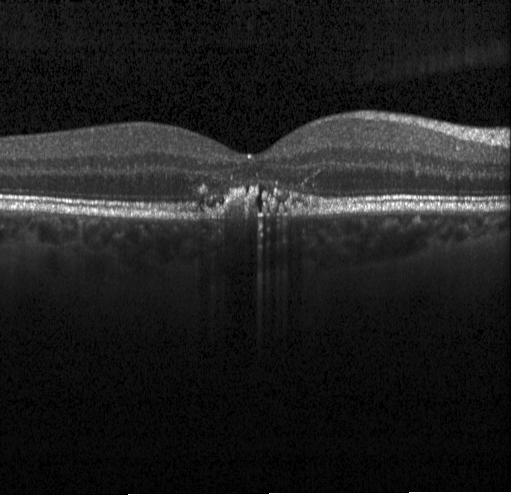

Optical coherence tomography B-scan. Assessment: choroidal neovascularization.